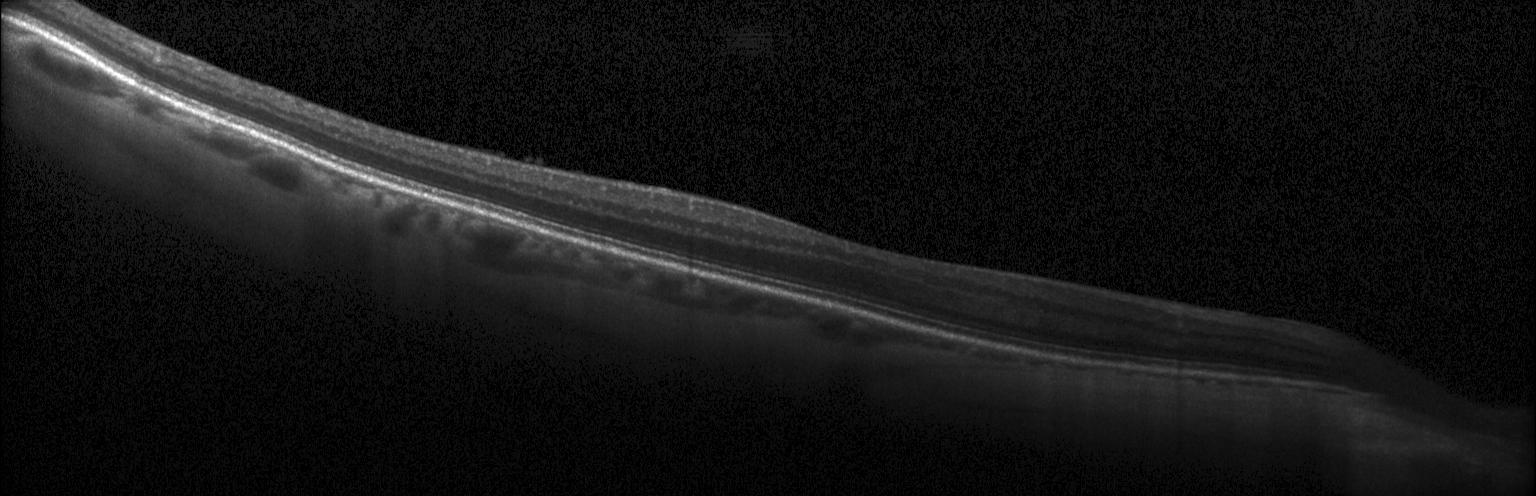 Assessment: no choroidal neovascularization, diabetic macular edema, or drusen.